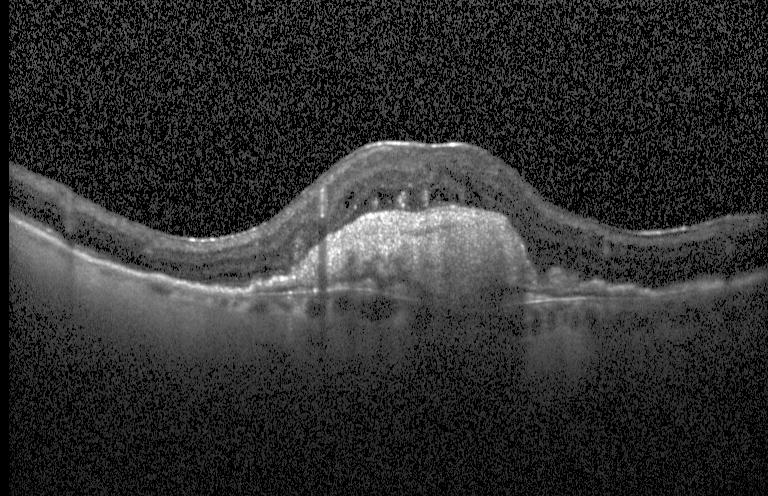

Acquired on a Heidelberg Spectralis. Spectral-domain optical coherence tomography. Horizontal scan through the fovea. Retinal OCT cross-section. Diagnosis: a choroidal neovascular membrane.